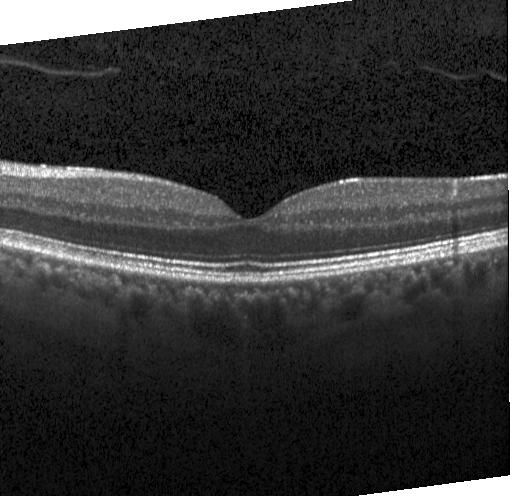 Optical coherence tomography B-scan — The scan shows no CNV, DME, or drusen.